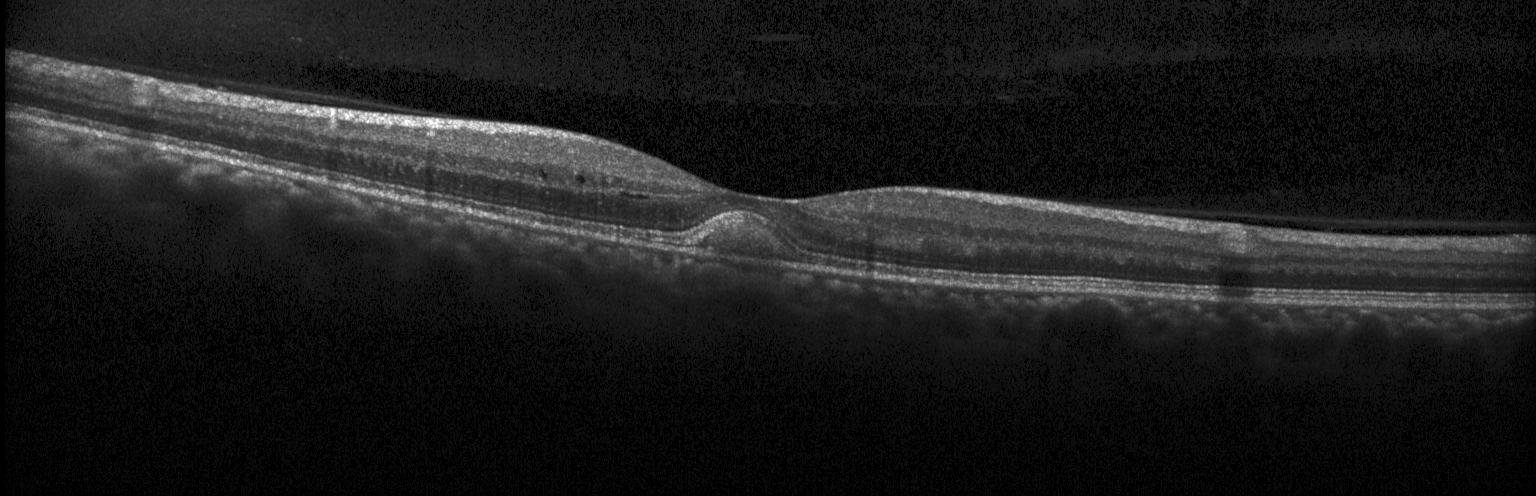

A choroidal neovascular membrane.